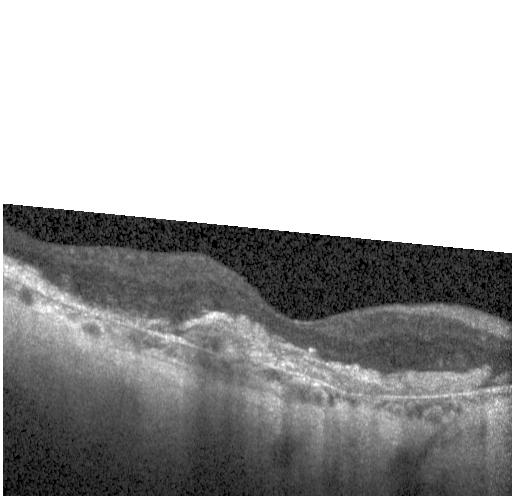
Spectral-domain OCT B-scan: a choroidal neovascular membrane.